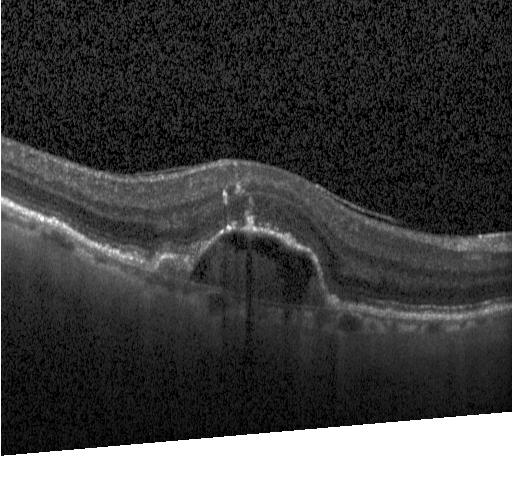
Retinal OCT B-scan
Finding: CNV.